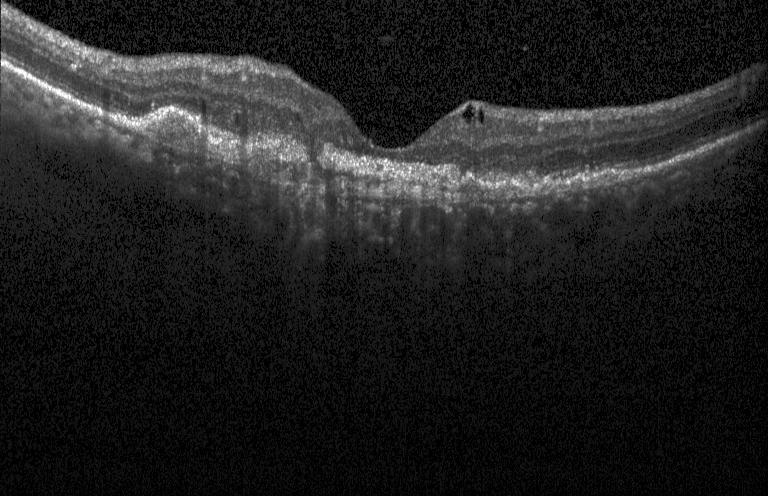 OCT line scan.
Assessment: a choroidal neovascular membrane.